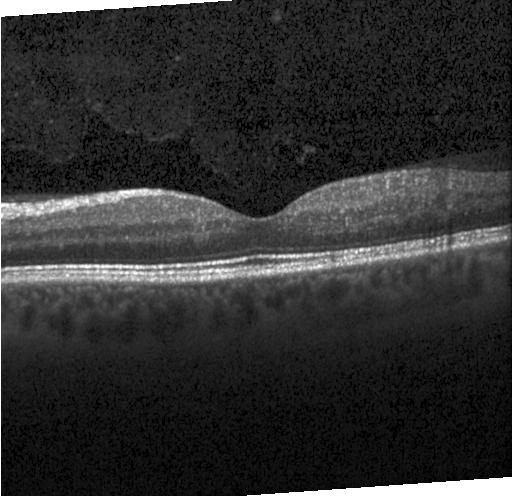
Retinal OCT cross-section showing neither CNV, DME, nor drusen.